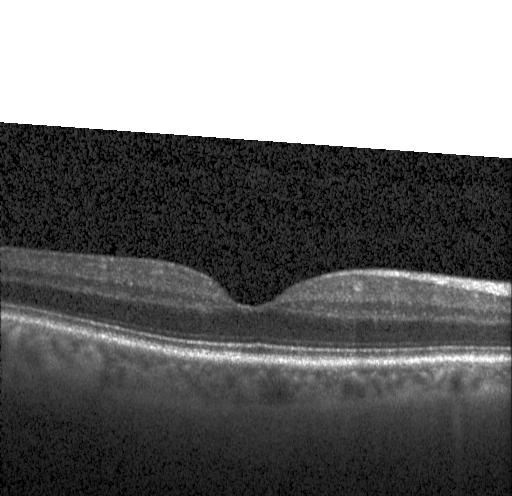
Finding: no CNV, DME, or drusen.